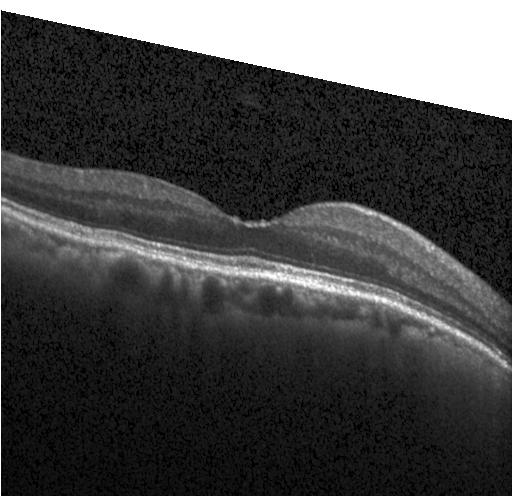
Retinal OCT cross-section. Horizontal scan through the fovea. Acquired on a Heidelberg Spectralis. SD-OCT. No CNV, no DME, and no drusen.